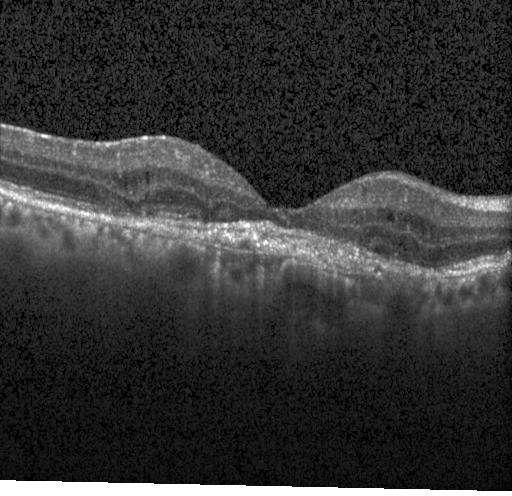
Retinal OCT B-scan — The scan shows a choroidal neovascular membrane.